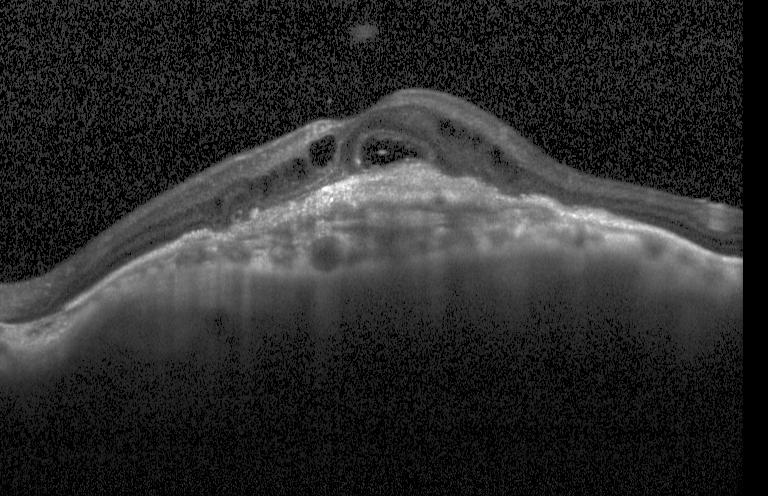

OCT scan showing CNV.